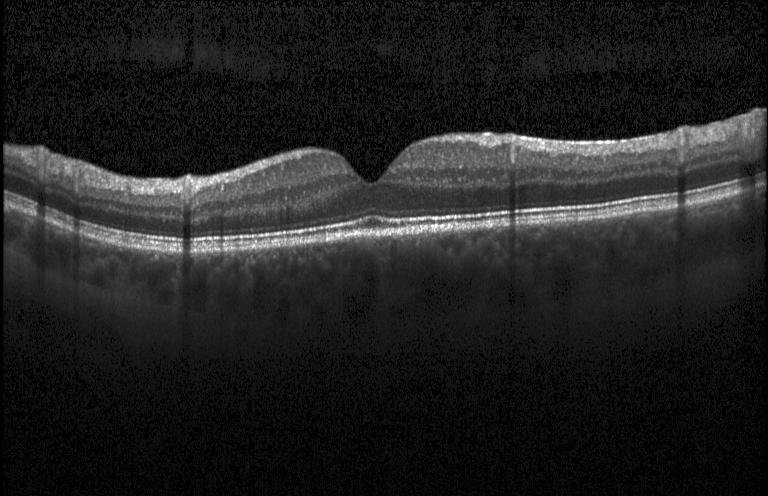
Spectral-domain optical coherence tomography · retinal OCT cross-section · instrument: Heidelberg Spectralis · through the macula. Diagnosis: no choroidal neovascularization, no diabetic macular edema, and no drusen.